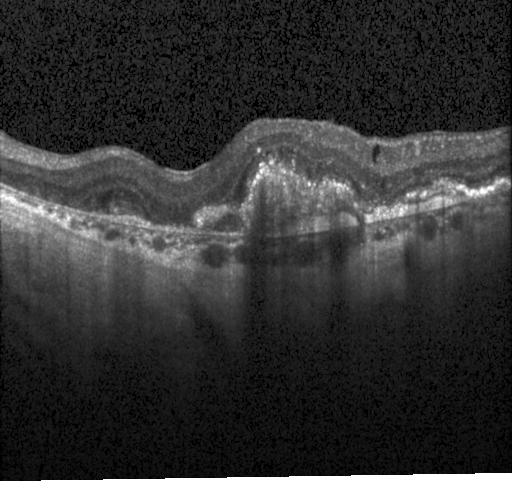

SD-OCT, OCT B-scan, Heidelberg Spectralis OCT system — This B-scan demonstrates choroidal neovascularization.